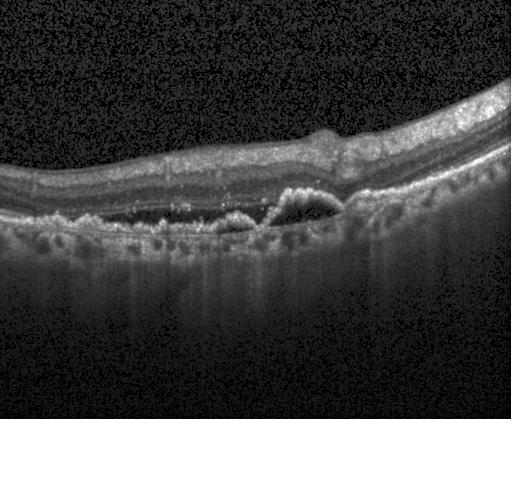
Retinal OCT B-scan — Diagnosis: a choroidal neovascular membrane.